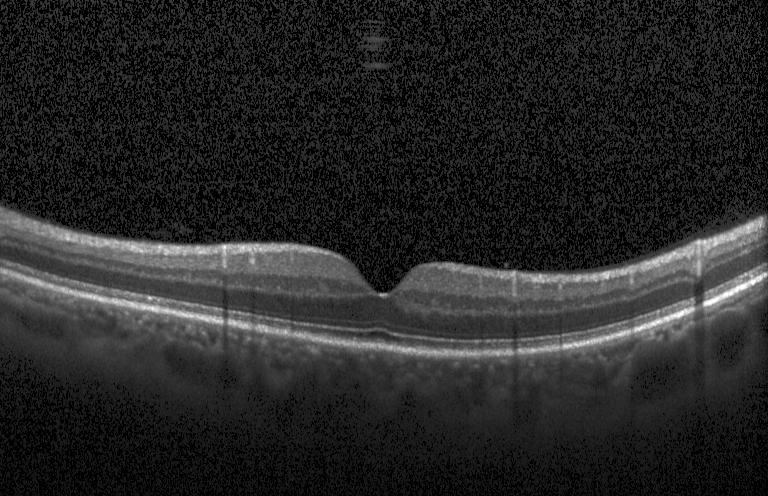 SD-OCT, through the macula, retinal OCT cross-section — Macular OCT: no CNV, no DME, and no drusen.